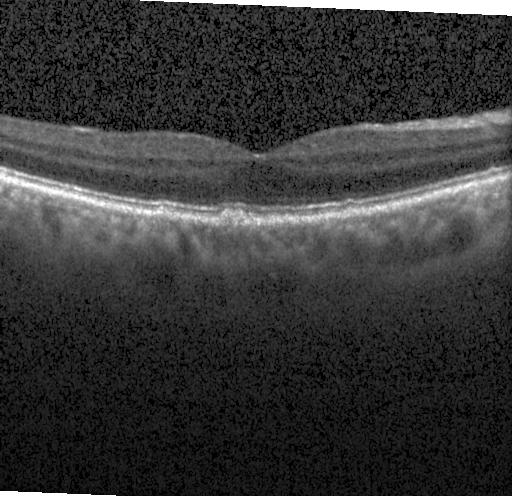
Retinal OCT cross-section · through the macula. Assessment: sub-RPE drusenoid deposits.